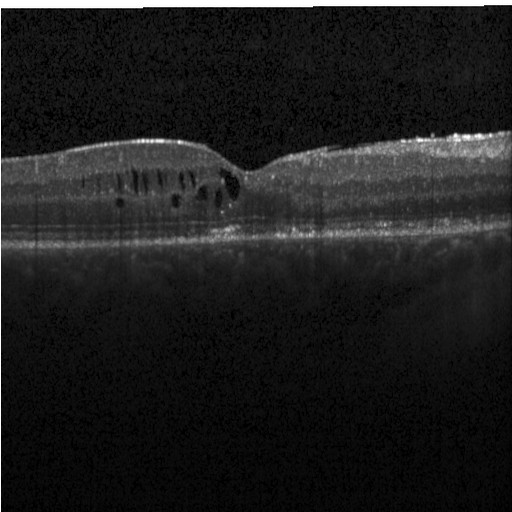

Dx: diabetic macular edema.